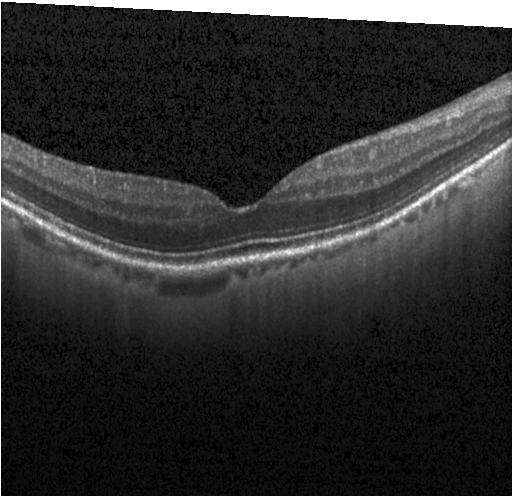 SD-OCT · OCT B-scan — No evidence of choroidal neovascularization, diabetic macular edema, or drusen.